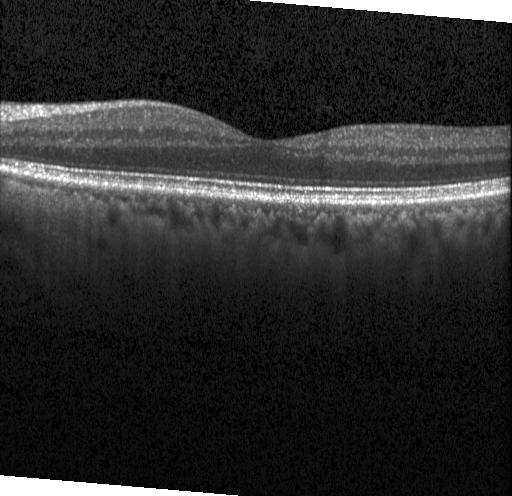

Finding: neither CNV, DME, nor drusen.